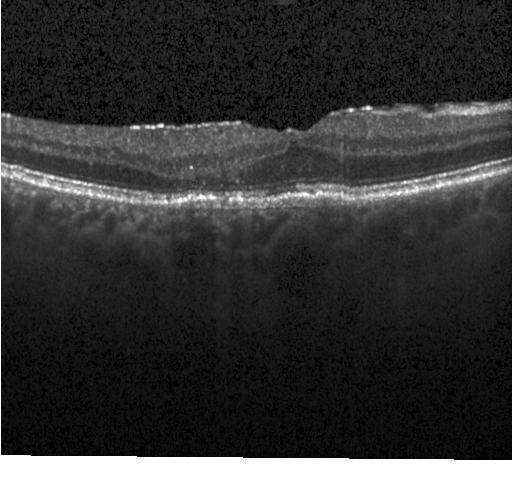 Horizontal scan through the fovea. Spectral-domain optical coherence tomography. Optical coherence tomography scan
Assessment: a choroidal neovascular membrane.